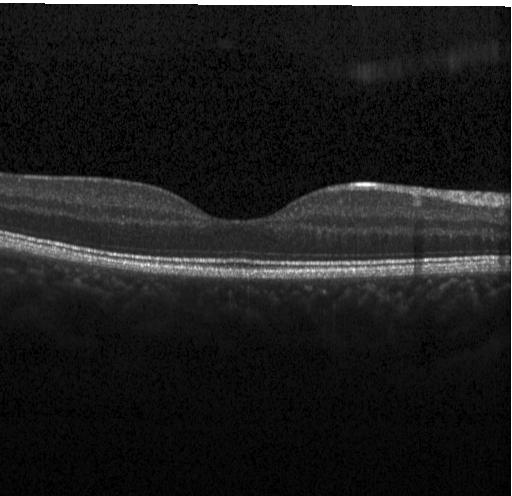 Retinal OCT cross-section.
Assessment: neither choroidal neovascularization, diabetic macular edema, nor drusen.